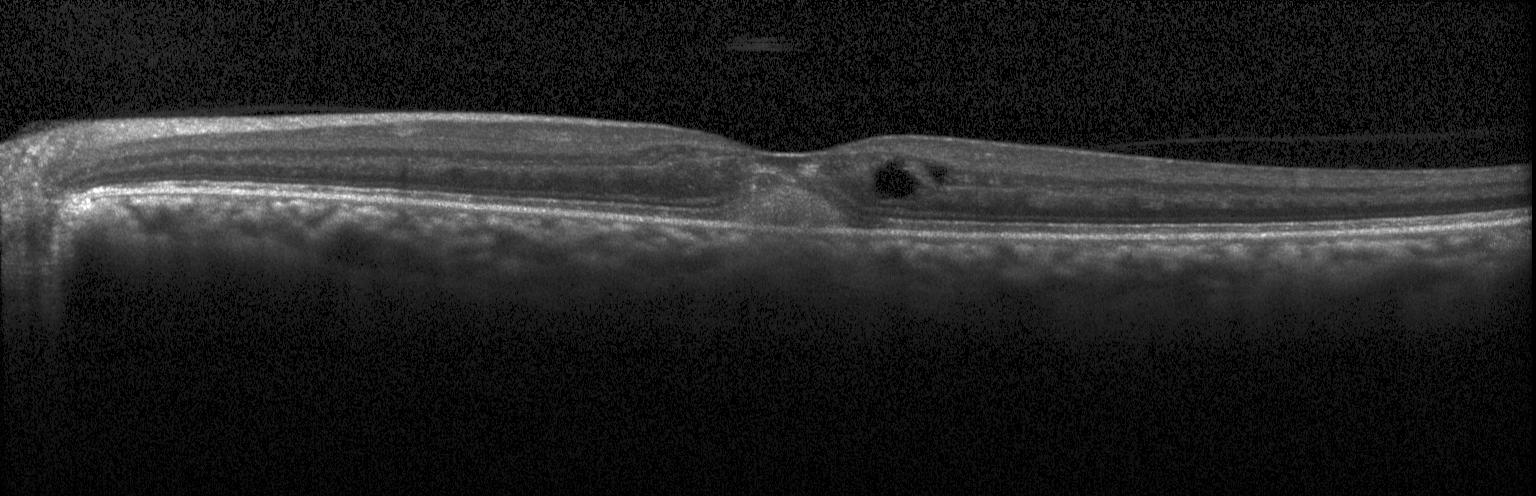 Macular scan · OCT B-scan · instrument: Heidelberg Spectralis. A choroidal neovascular membrane.